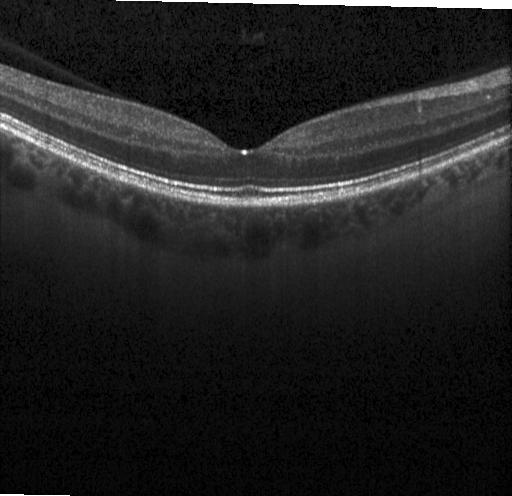
Retinal OCT cross-section, horizontal scan through the fovea.
Diagnosis: no evidence of CNV, DME, or drusen.